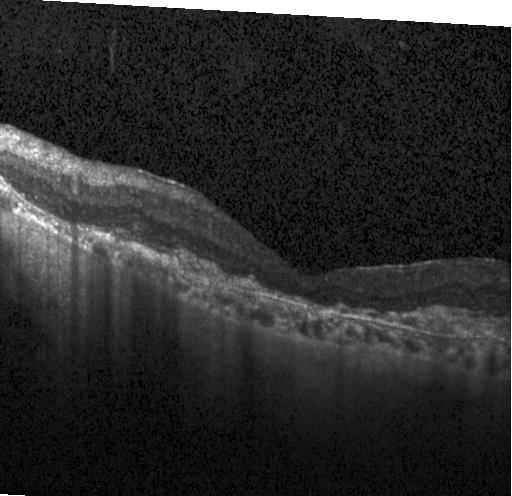

OCT line scan
OCT finding: choroidal neovascularization.